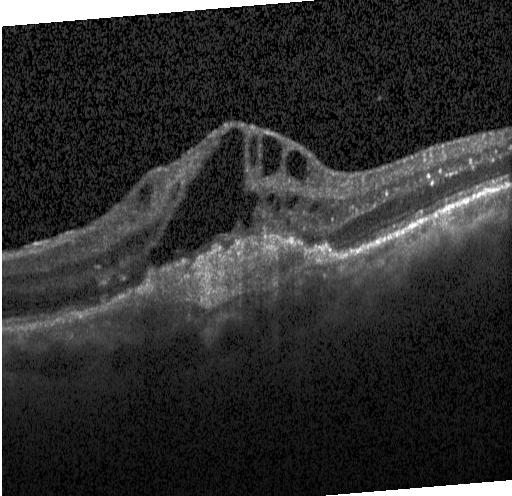
SD-OCT; optical coherence tomography B-scan; Heidelberg Spectralis.
Macular OCT: a choroidal neovascular membrane.